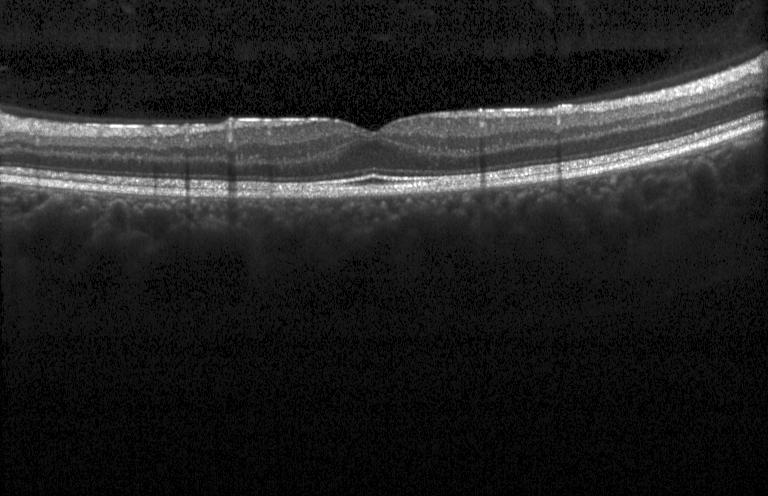
Macular OCT demonstrating no choroidal neovascularization, no diabetic macular edema, and no drusen.